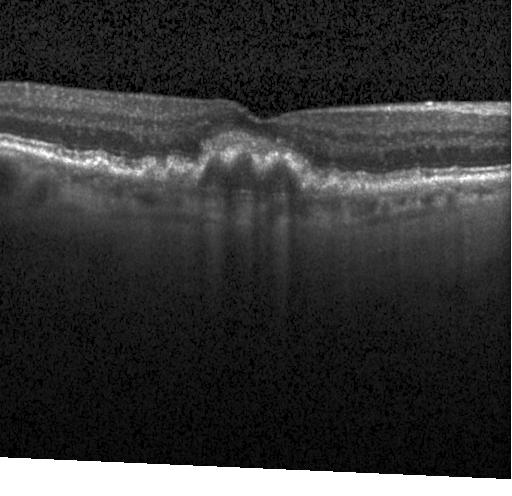 The scan shows choroidal neovascularization.